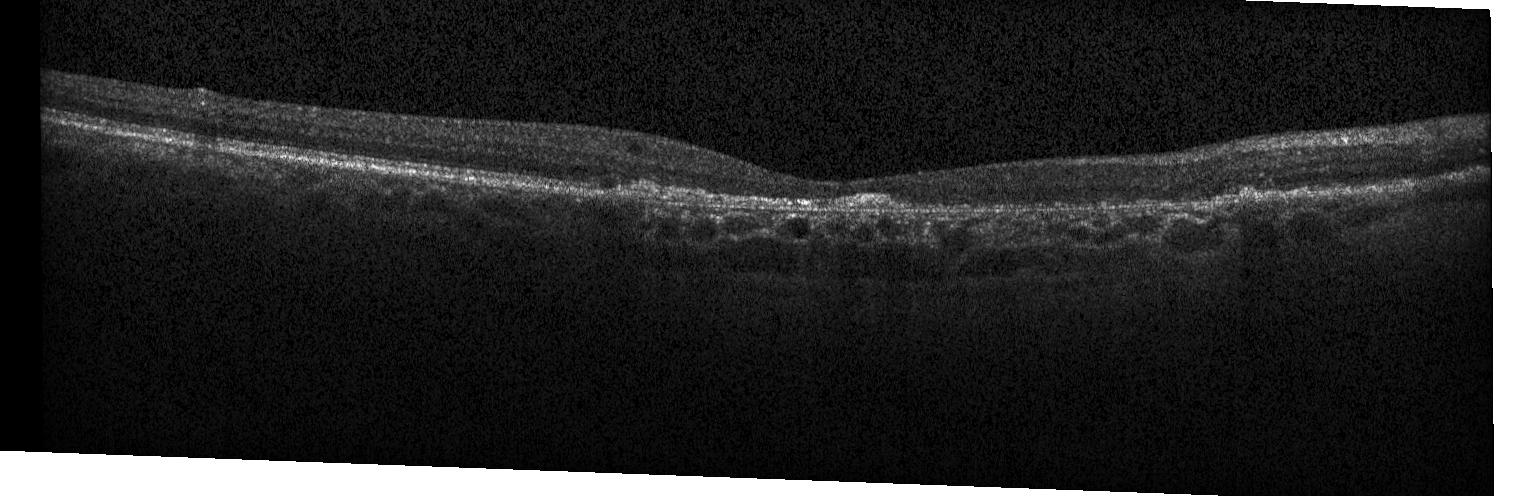 Retinal OCT B-scan. OCT finding: a choroidal neovascular membrane.